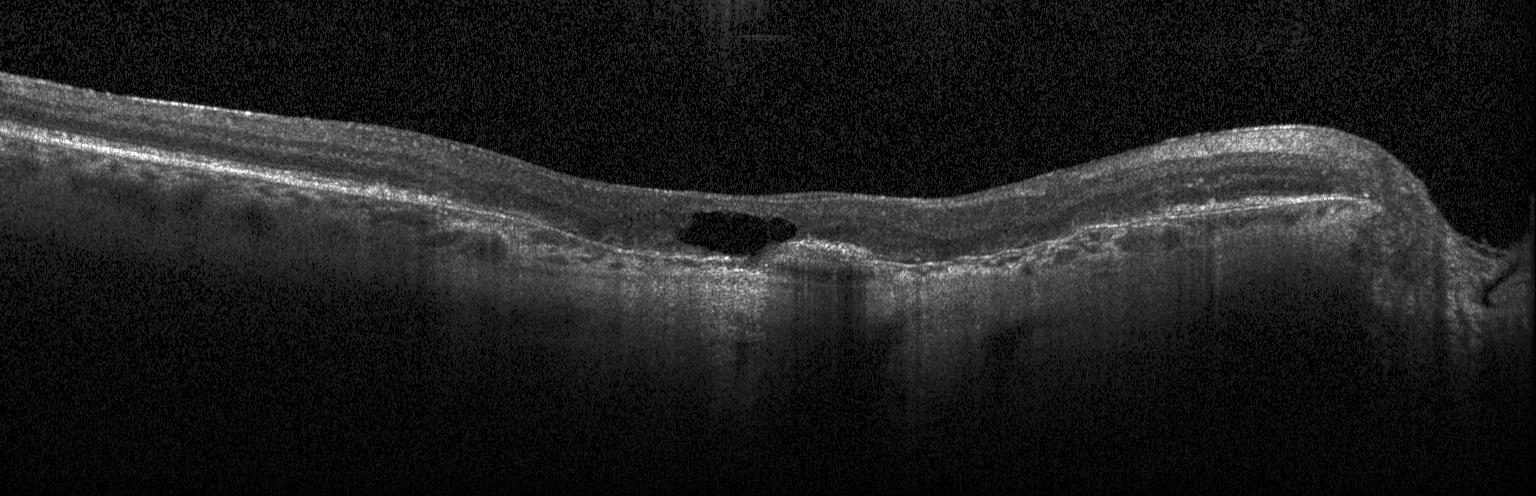
Optical coherence tomography B-scan.
Macular OCT: a choroidal neovascular membrane.